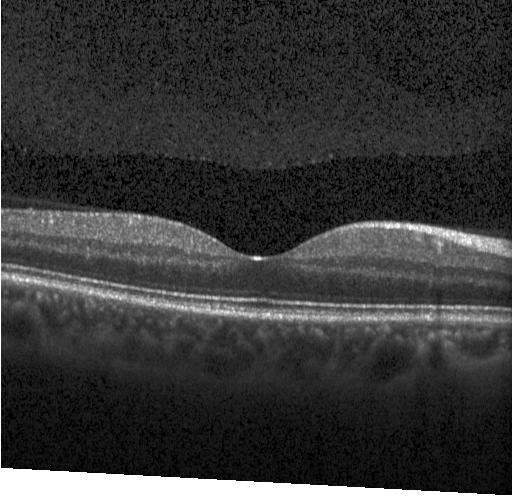
Retinal OCT B-scan
Impression: neither choroidal neovascularization, diabetic macular edema, nor drusen.